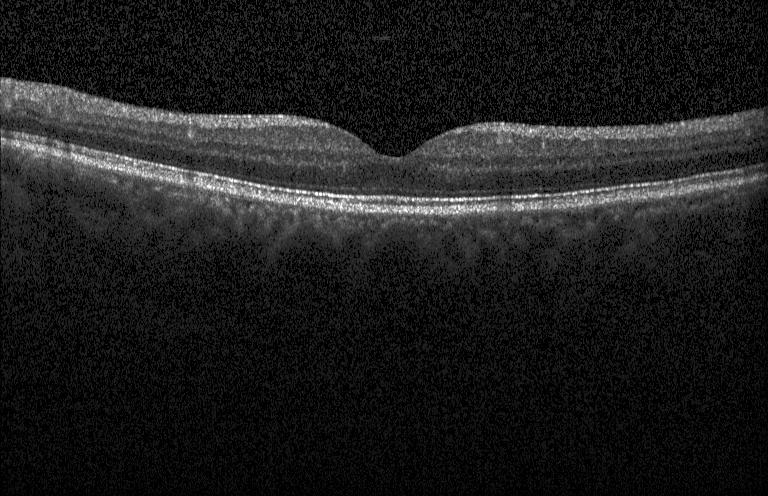 Fovea-centered · retinal OCT B-scan · SD-OCT.
The scan shows no choroidal neovascularization, no diabetic macular edema, and no drusen.